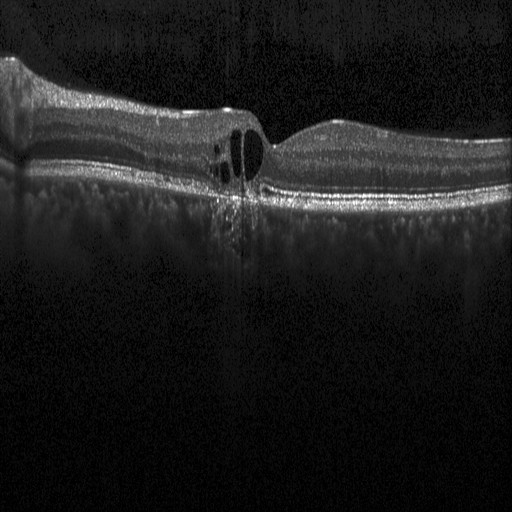
Spectral-domain OCT B-scan: diabetic macular edema (DME).